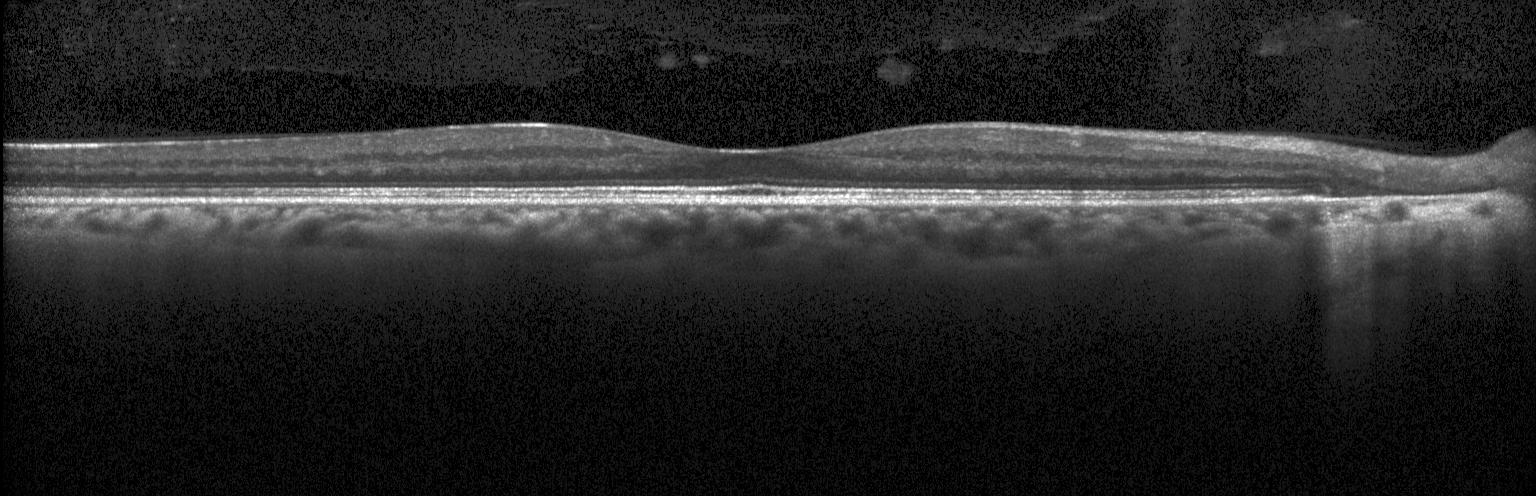 Finding: neither choroidal neovascularization, diabetic macular edema, nor drusen.